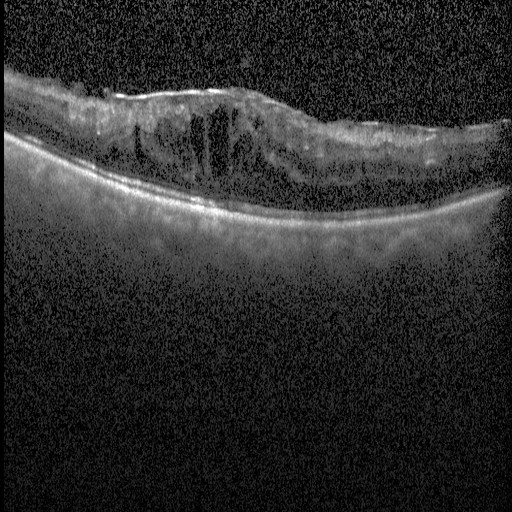 Optical coherence tomography scan, spectral-domain OCT, fovea-centered
Diabetic macular edema (DME).